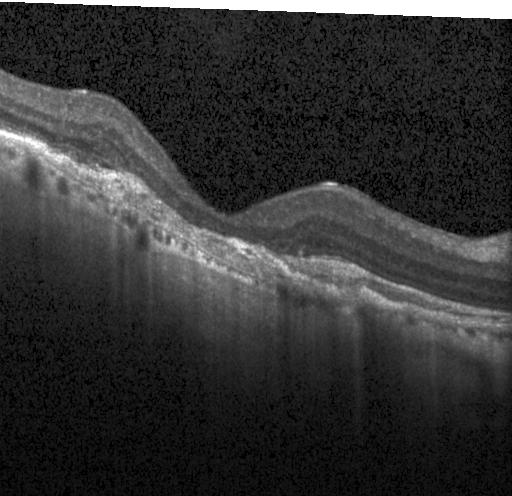 Heidelberg Spectralis OCT system; spectral-domain optical coherence tomography; fovea-centered; OCT line scan. The scan shows CNV.